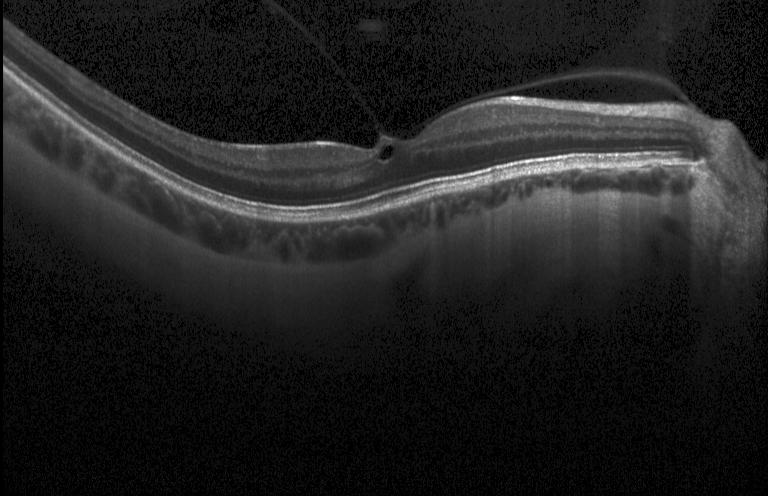
Retinal OCT cross-section showing neither choroidal neovascularization, diabetic macular edema, nor drusen.